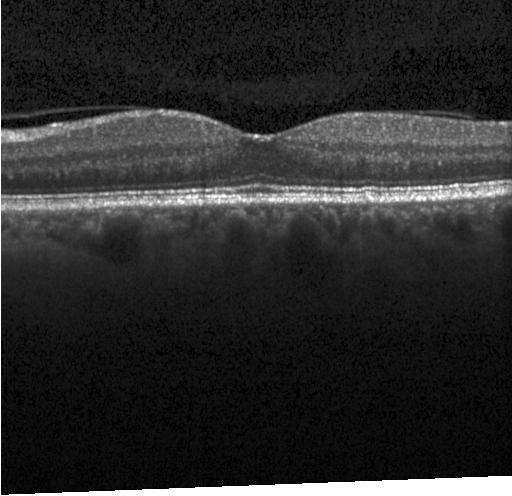

Diagnosis: no evidence of choroidal neovascularization, diabetic macular edema, or drusen.